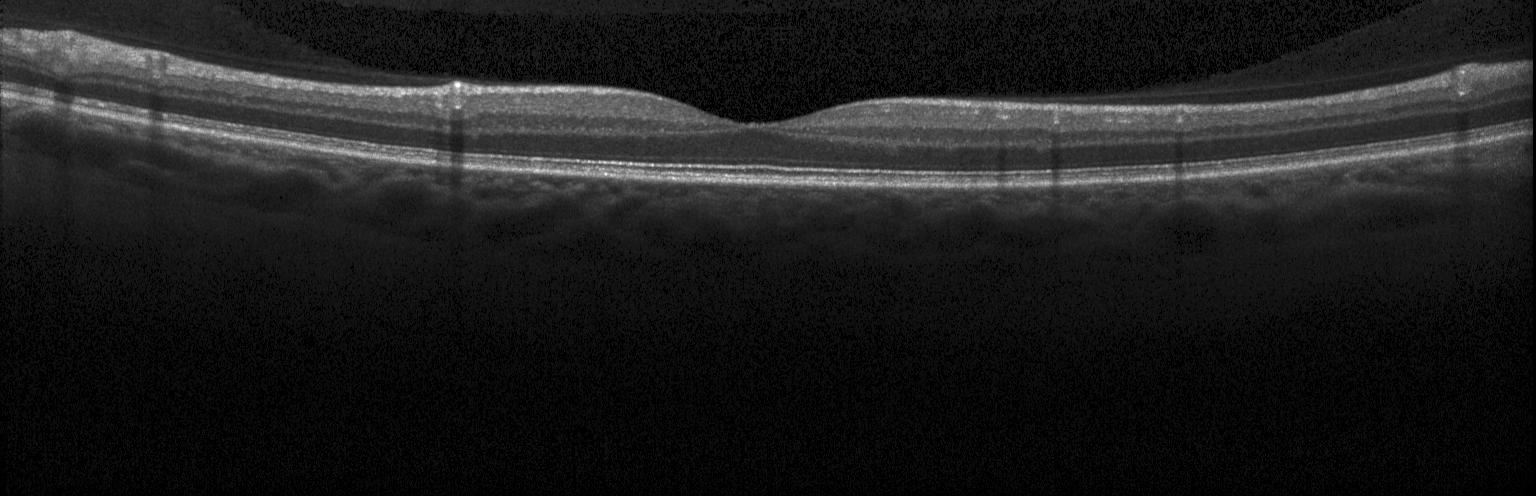
OCT B-scan showing no CNV, DME, or drusen.